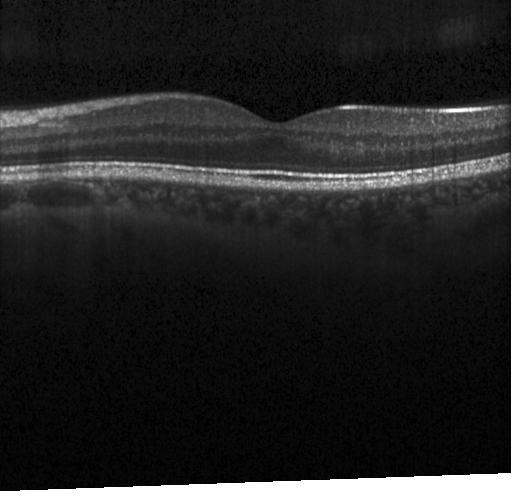

Diagnosis: no evidence of CNV, DME, or drusen.